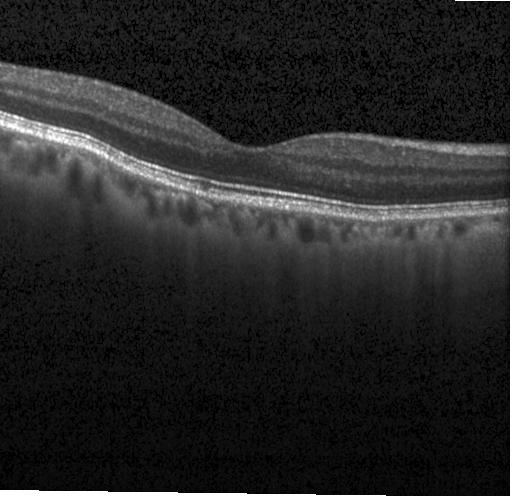 Retinal OCT B-scan.
Assessment: neither CNV, DME, nor drusen.